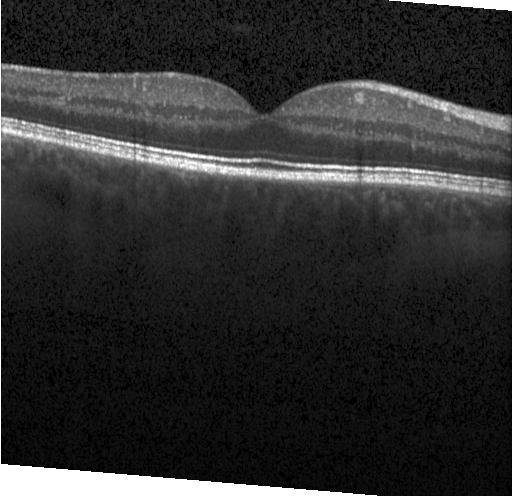 Macular scan, retinal OCT B-scan — Impression: no evidence of CNV, DME, or drusen.